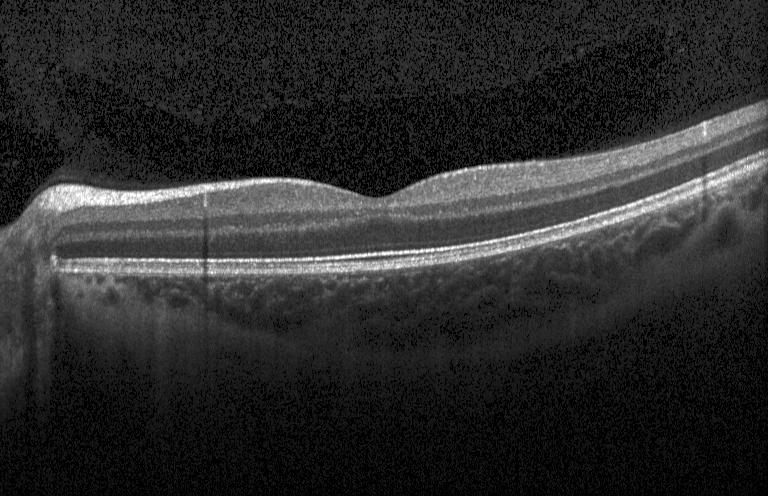 Optical coherence tomography B-scan, spectral-domain OCT. Finding: no evidence of choroidal neovascularization, diabetic macular edema, or drusen.